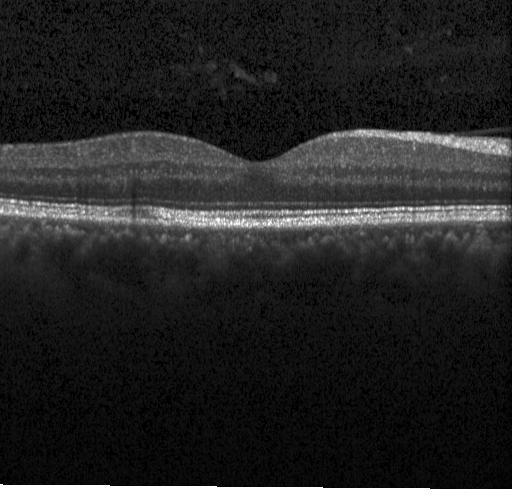
OCT B-scan — Impression: no evidence of choroidal neovascularization, diabetic macular edema, or drusen.